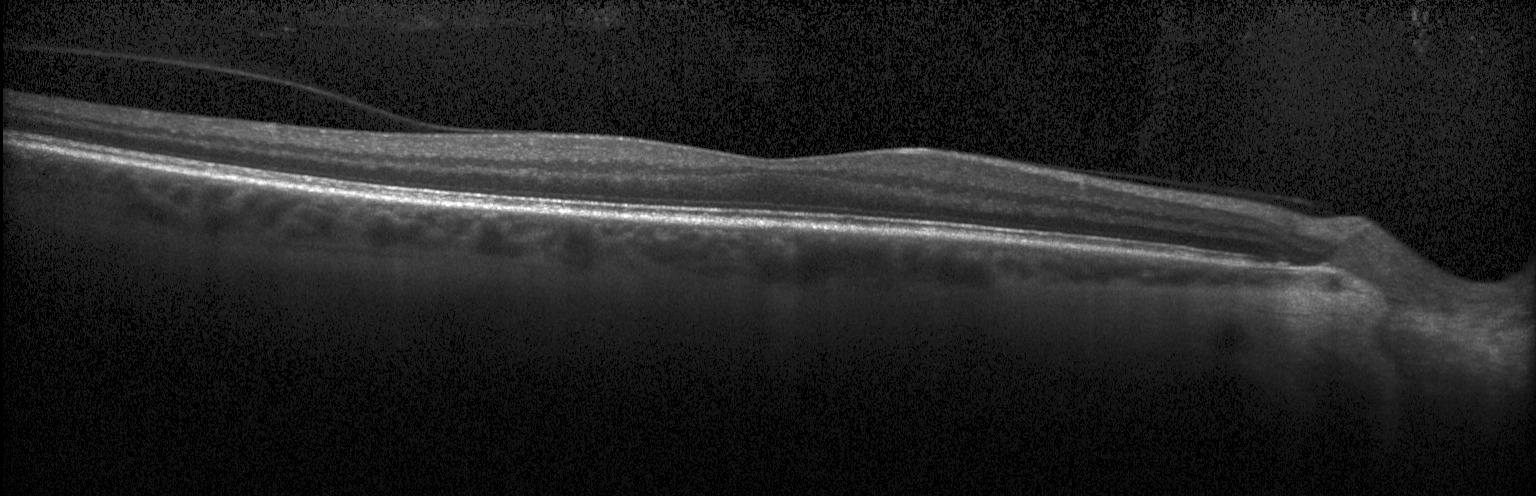

Optical coherence tomography scan
Assessment: neither choroidal neovascularization, diabetic macular edema, nor drusen.